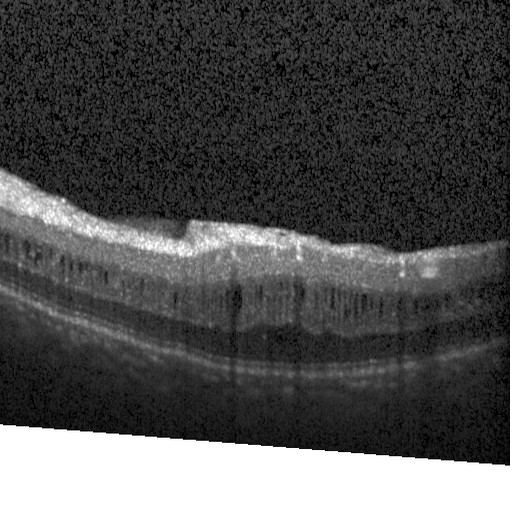 Macular OCT demonstrating diabetic macular edema (DME).